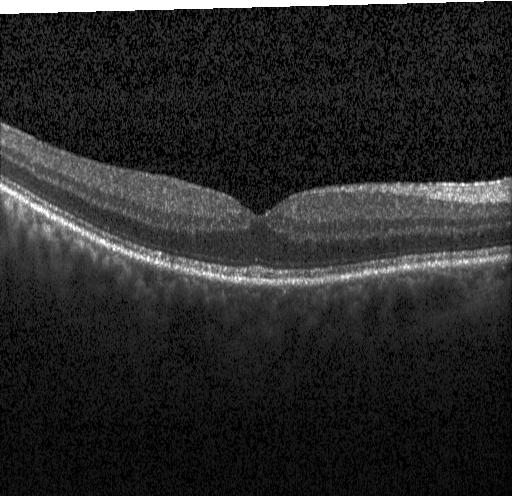

Through the macula; SD-OCT; acquired on a Heidelberg Spectralis; retinal OCT B-scan.
Impression: no evidence of choroidal neovascularization, diabetic macular edema, or drusen.